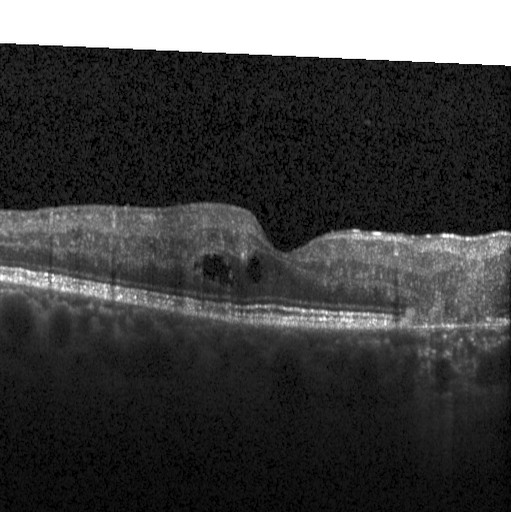 OCT finding: DME.